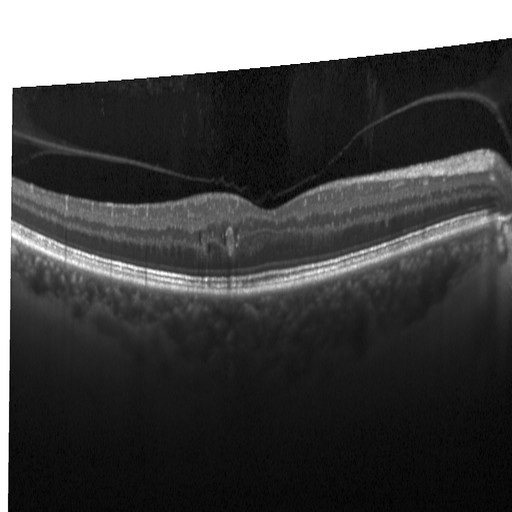
Acquired on a Heidelberg Spectralis, optical coherence tomography B-scan
Assessment: DME.